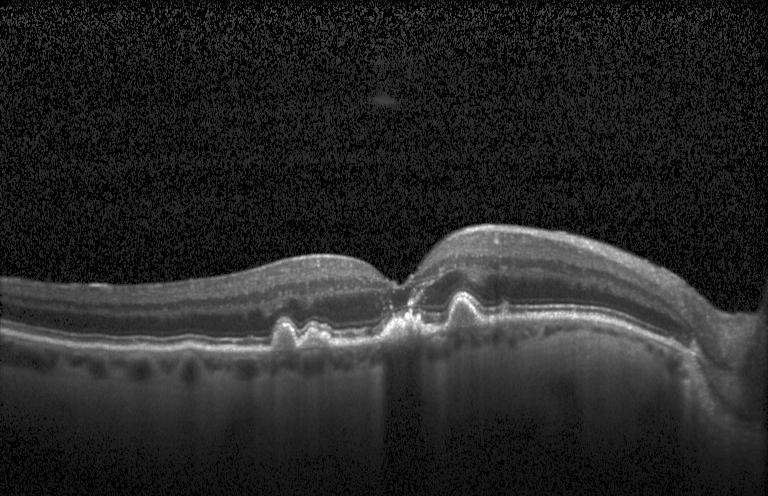
Acquired on a Heidelberg Spectralis; fovea-centered; optical coherence tomography scan; SD-OCT. Sub-RPE drusenoid deposits.